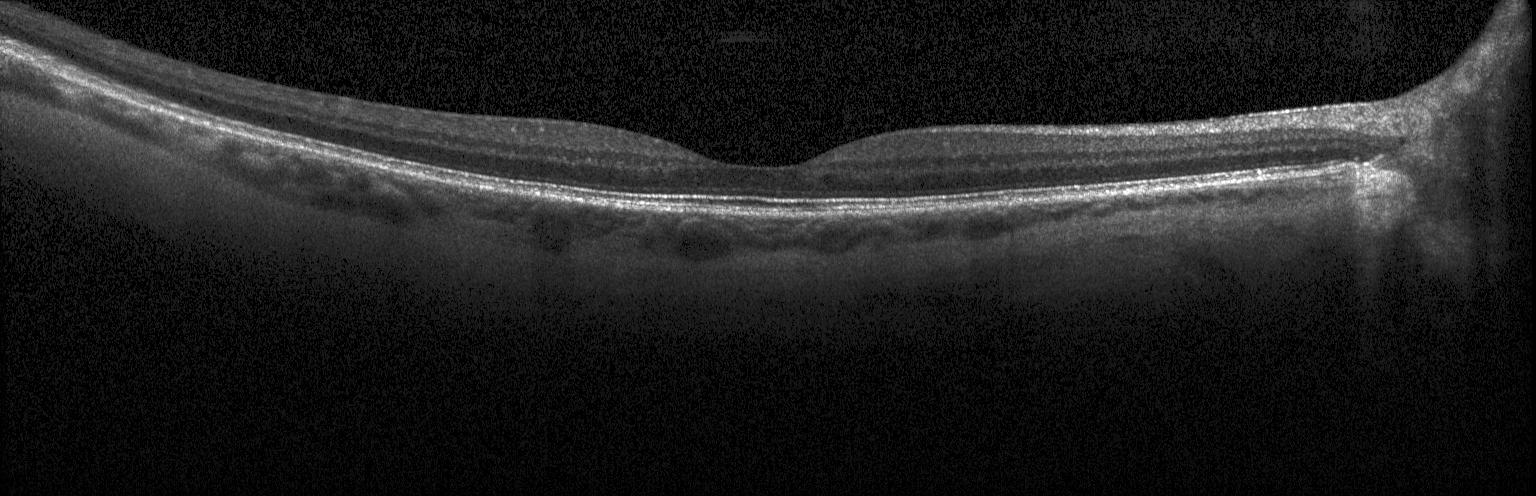

Retinal OCT cross-section — Finding: no evidence of choroidal neovascularization, diabetic macular edema, or drusen.